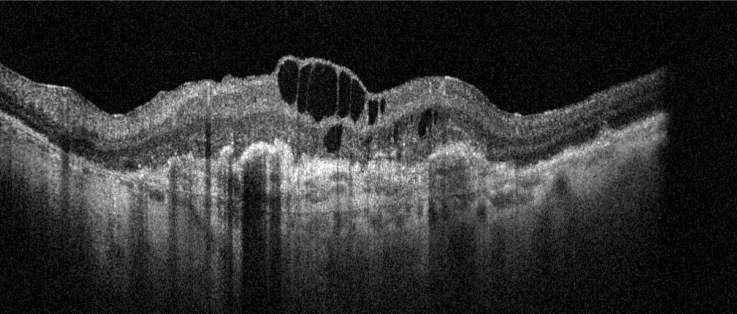
Optical coherence tomography B-scan — The scan shows AMD.